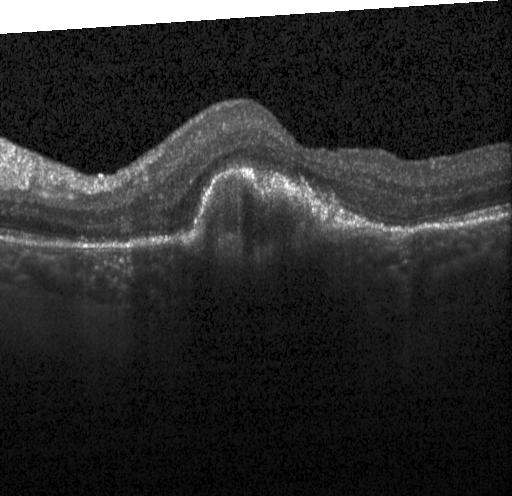 Spectral-domain optical coherence tomography. Acquired on a Heidelberg Spectralis. Retinal OCT cross-section. Finding: a choroidal neovascular membrane.